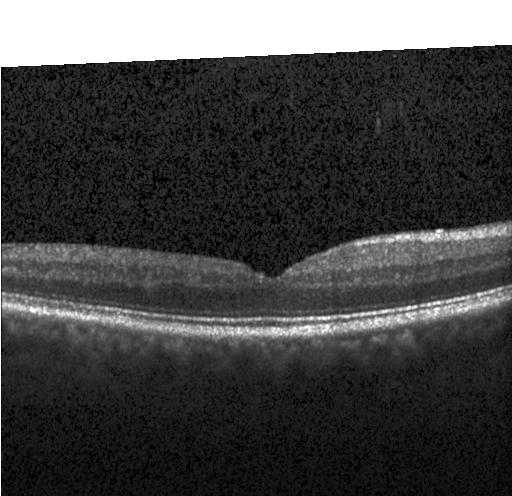
Impression: no evidence of choroidal neovascularization, diabetic macular edema, or drusen.